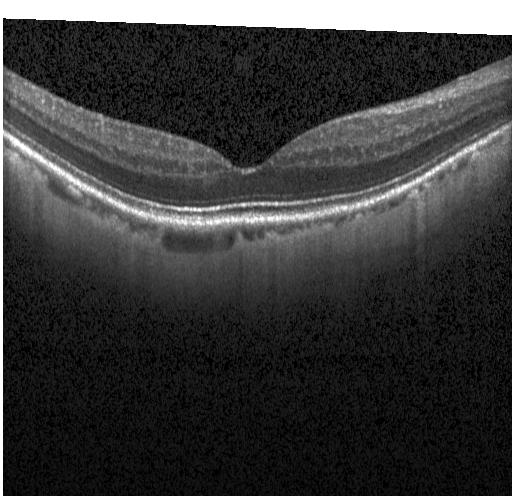 OCT scan showing no choroidal neovascularization, no diabetic macular edema, and no drusen.